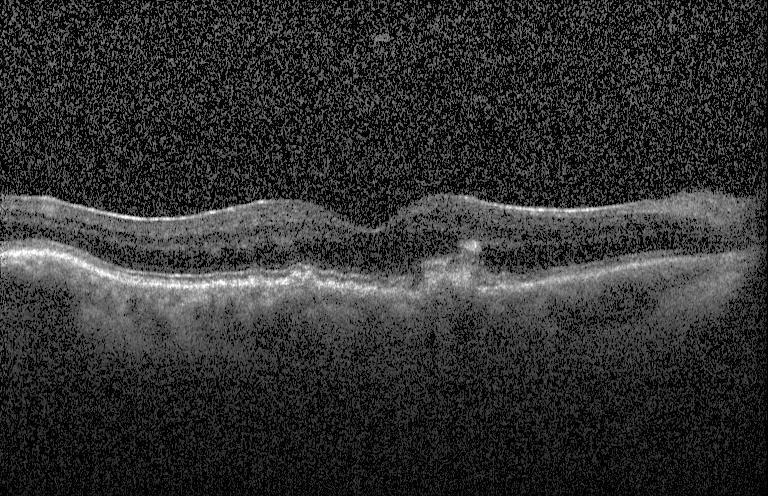 Retinal OCT cross-section · fovea-centered · SD-OCT · Heidelberg Spectralis
OCT finding: multiple drusen.